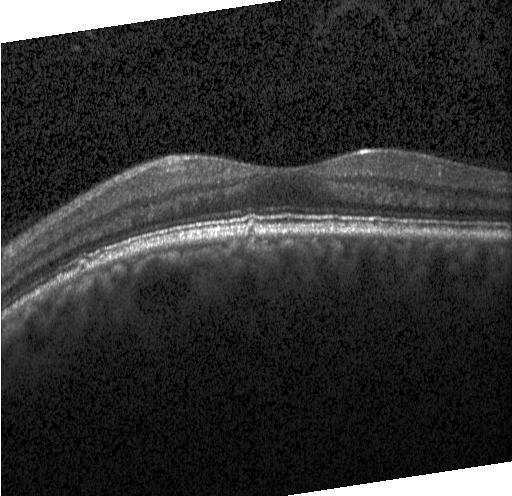 Heidelberg Spectralis OCT system, retinal OCT B-scan, through the macula, spectral-domain OCT.
The scan shows multiple drusen.